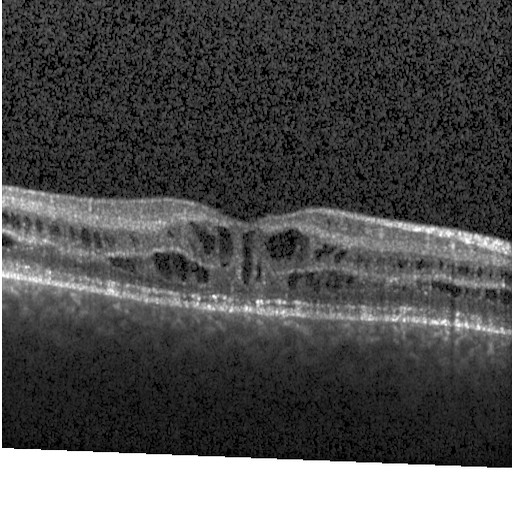

OCT B-scan
This B-scan demonstrates diabetic macular edema (DME).